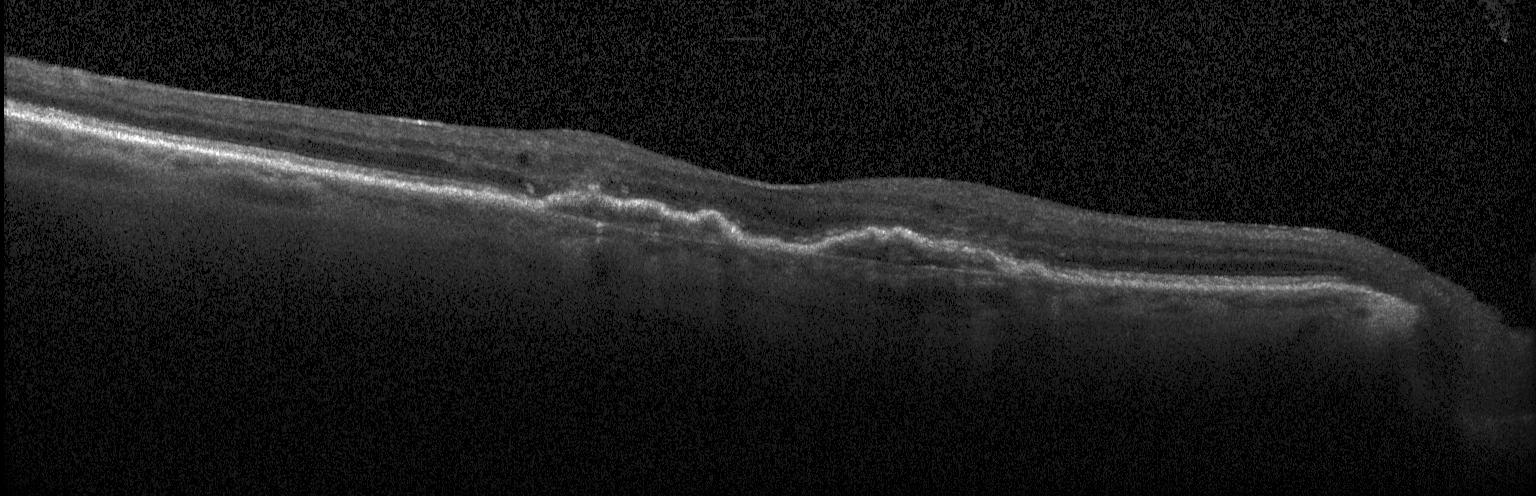 Diagnosis: choroidal neovascularization.